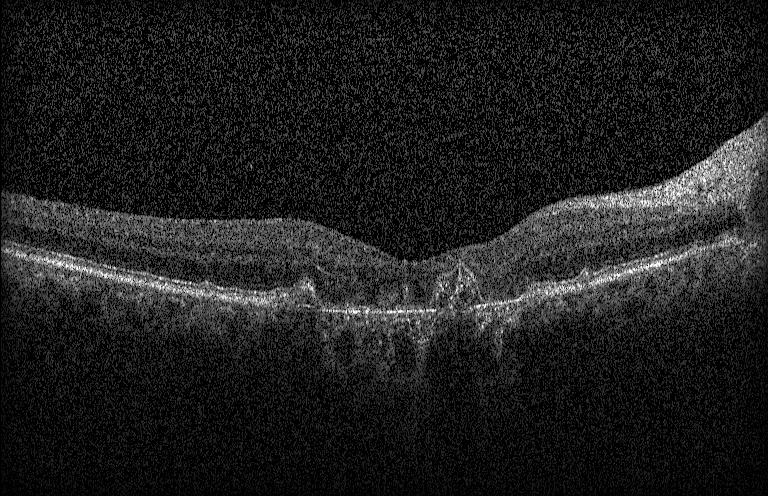 OCT B-scan showing a choroidal neovascular membrane.